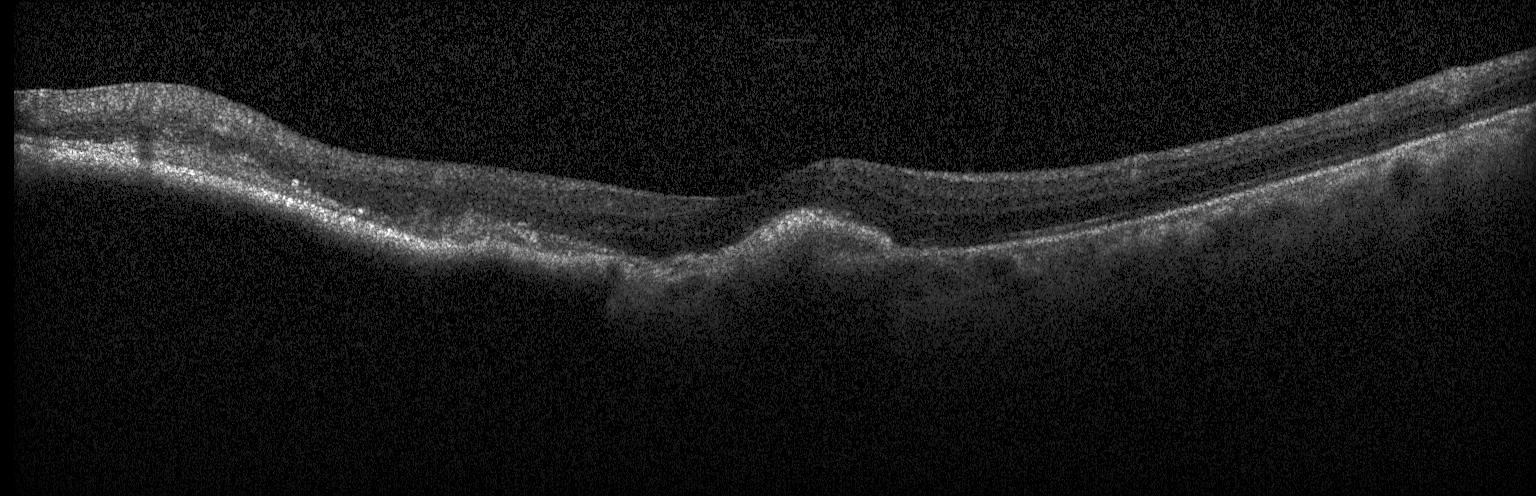

Assessment: CNV.